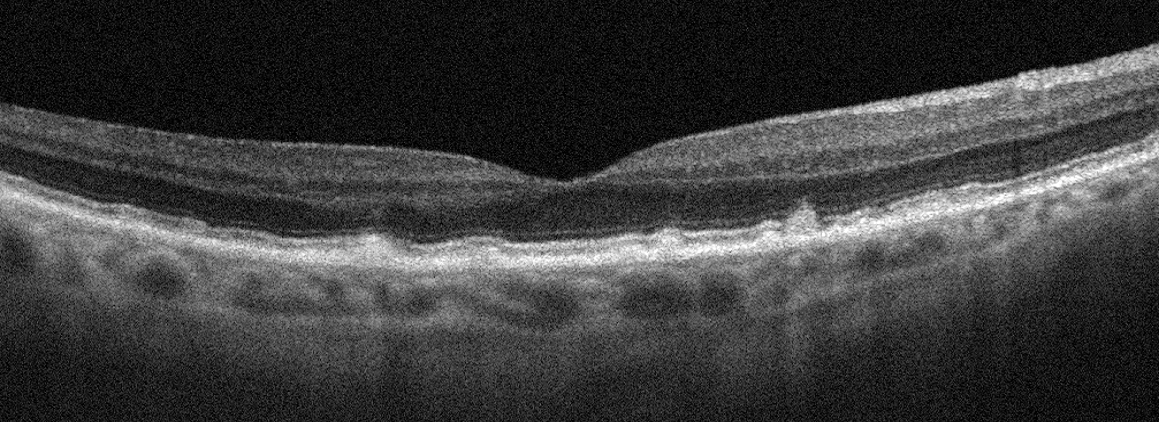 OCT B-scan; OD.
This B-scan demonstrates age-related macular degeneration (AMD).